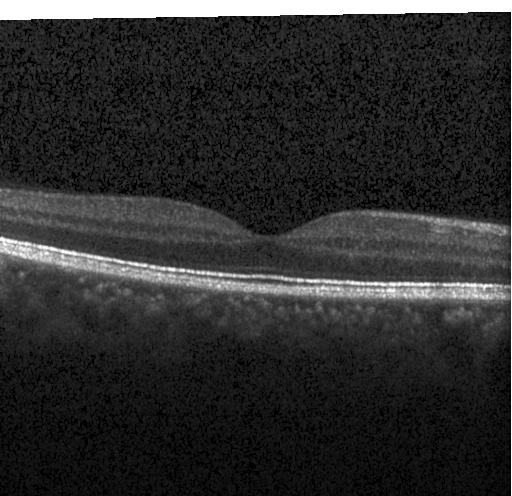
Finding: neither CNV, DME, nor drusen.